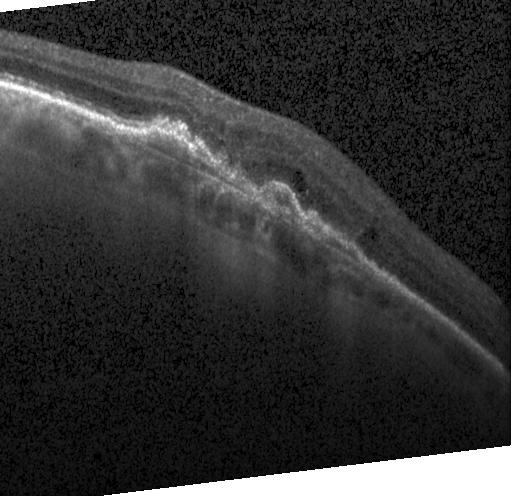

Macular OCT: a choroidal neovascular membrane.